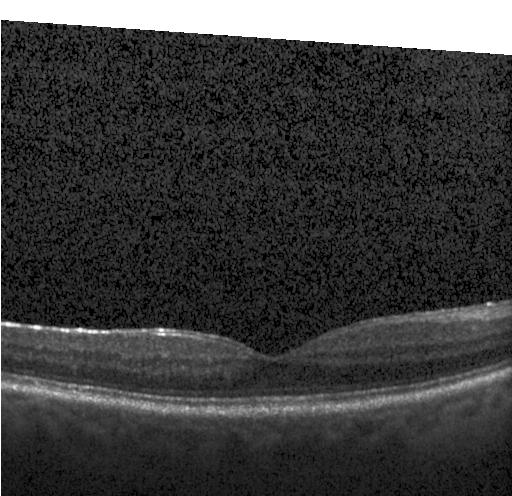
Retinal OCT cross-section.
The scan shows no CNV, DME, or drusen.